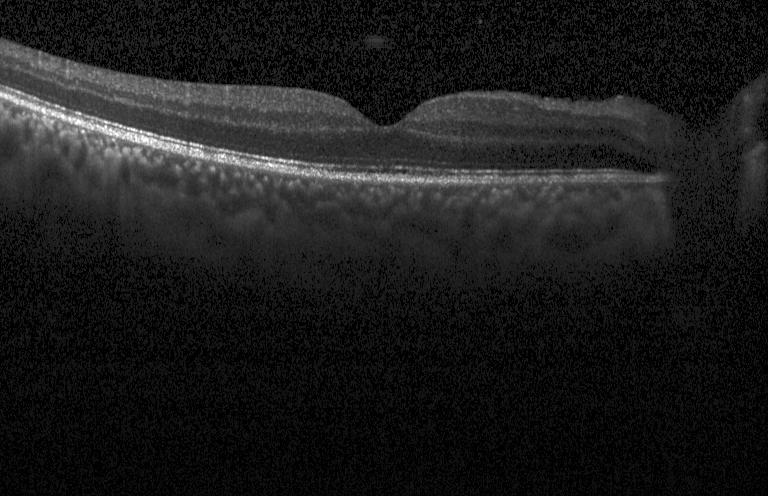 The scan shows no choroidal neovascularization, no diabetic macular edema, and no drusen.